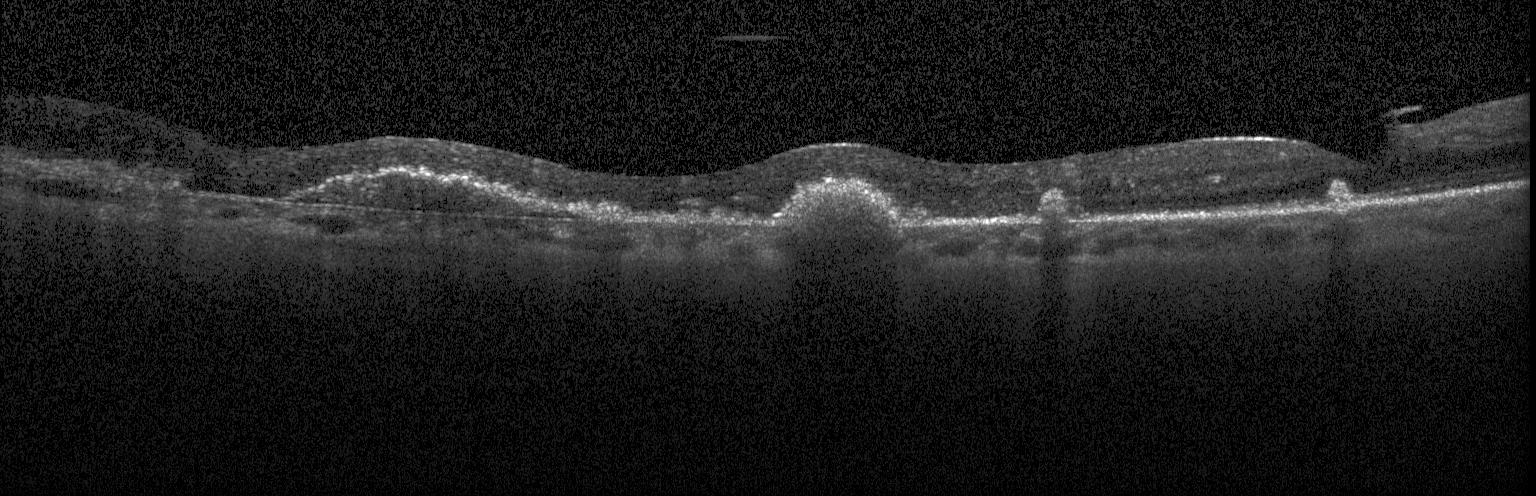
OCT B-scan · horizontal scan through the fovea.
Diagnosis: choroidal neovascularization.